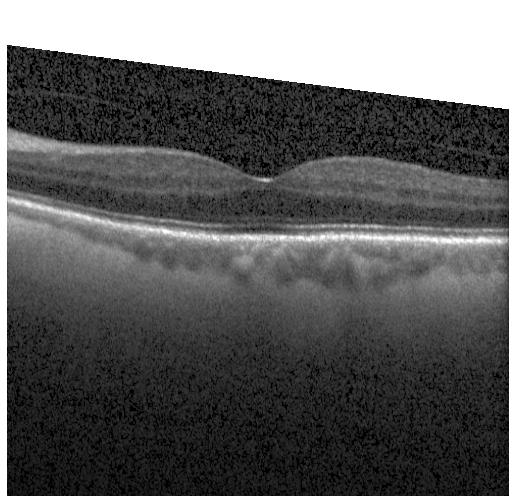

Macular scan. Retinal OCT cross-section. Acquired on a Heidelberg Spectralis — Diagnosis: no choroidal neovascularization, no diabetic macular edema, and no drusen.